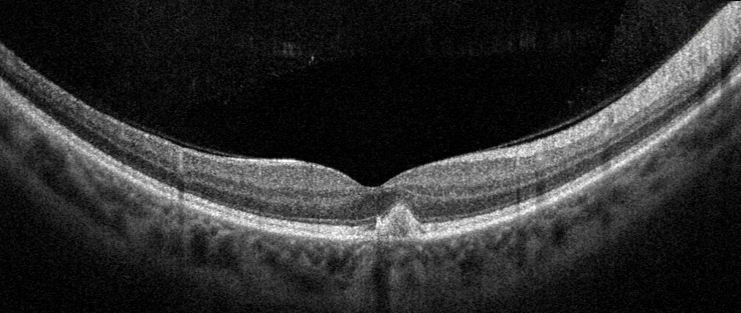 OCT line scan. Macular OCT: AMD.